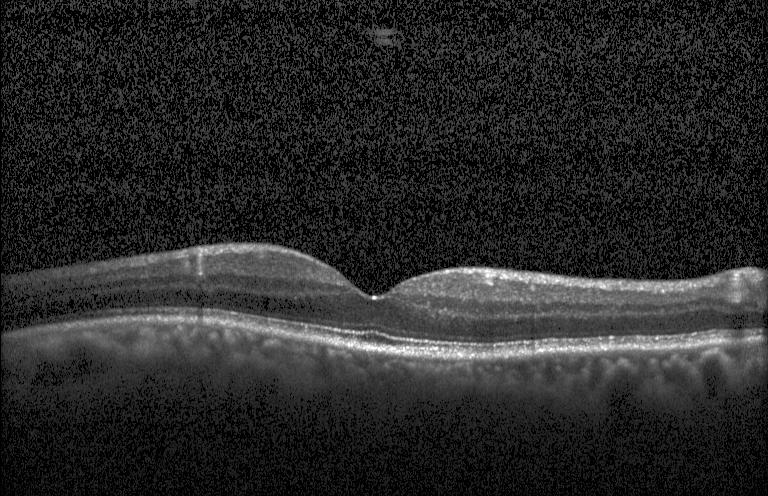
Heidelberg Spectralis; spectral-domain optical coherence tomography; optical coherence tomography B-scan; macular scan — Impression: no CNV, DME, or drusen.